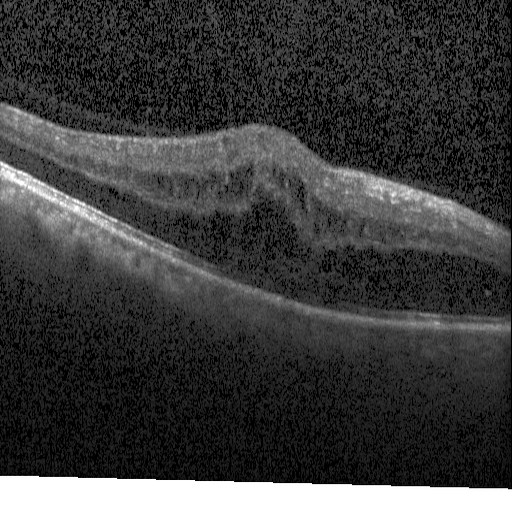

Dx: diabetic macular edema.